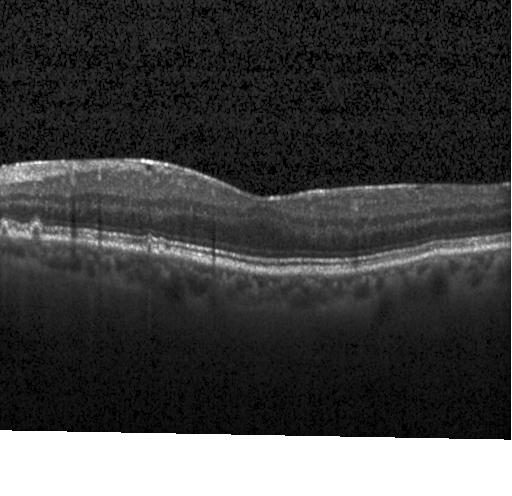 Diagnosis: drusen.